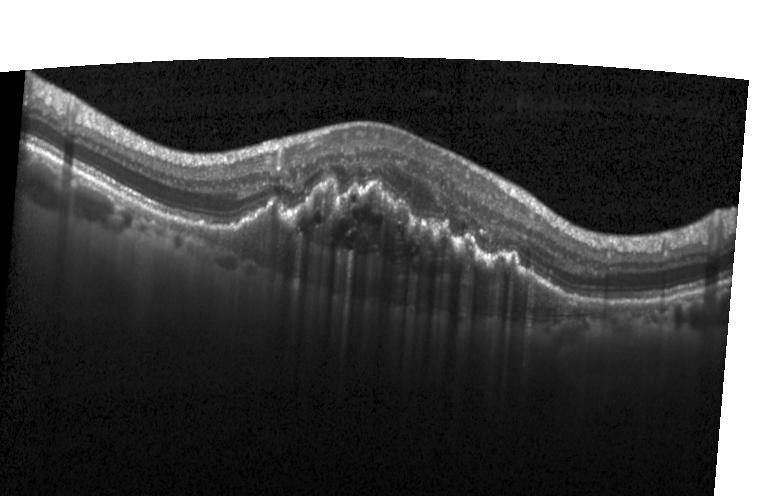
OCT B-scan, Heidelberg Spectralis — Impression: CNV.